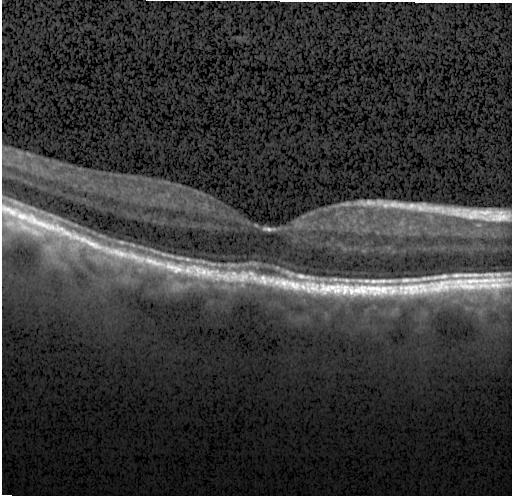
OCT line scan. Impression: no evidence of choroidal neovascularization, diabetic macular edema, or drusen.